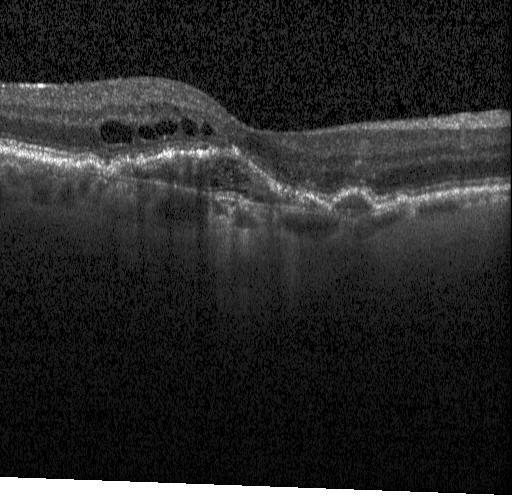
Horizontal scan through the fovea, SD-OCT, optical coherence tomography B-scan — Diagnosis: choroidal neovascularization (CNV).